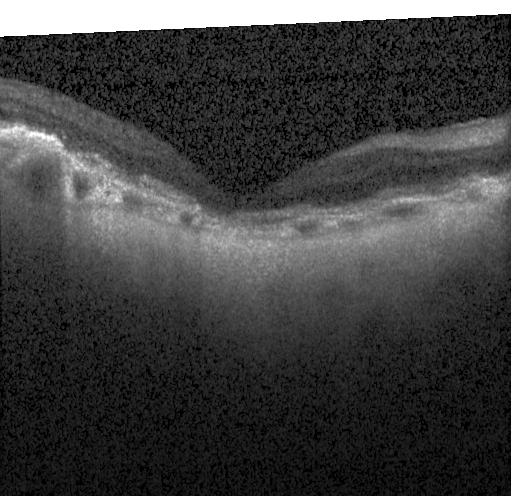

Heidelberg Spectralis, retinal OCT cross-section
Finding: a choroidal neovascular membrane.